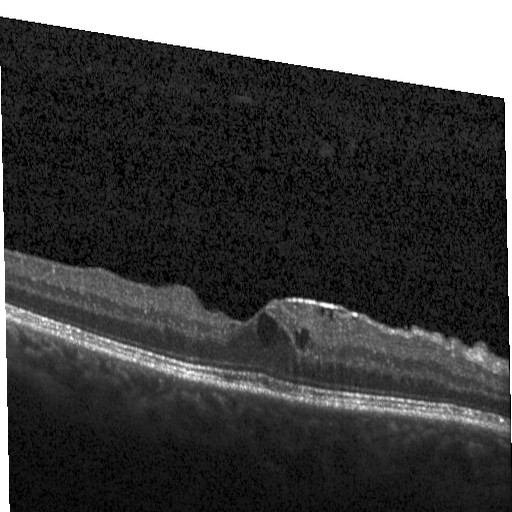
Spectral-domain OCT, instrument: Heidelberg Spectralis, optical coherence tomography scan. Impression: diabetic macular edema (DME).